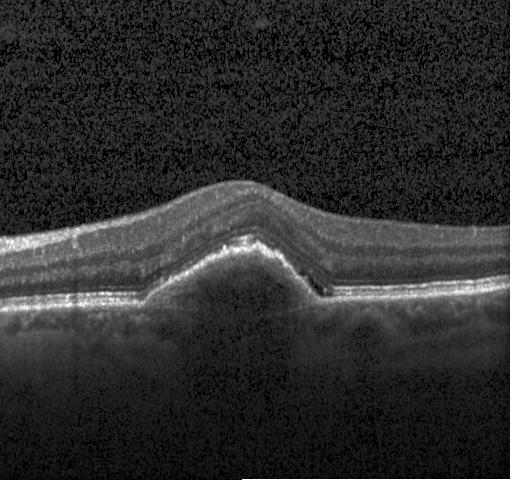

Centered on the fovea; optical coherence tomography scan
Diagnosis: choroidal neovascularization.